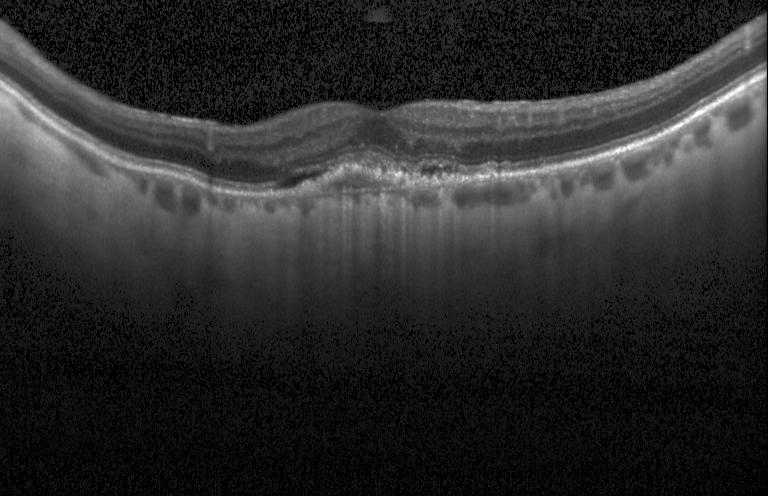

Assessment: choroidal neovascularization (CNV).